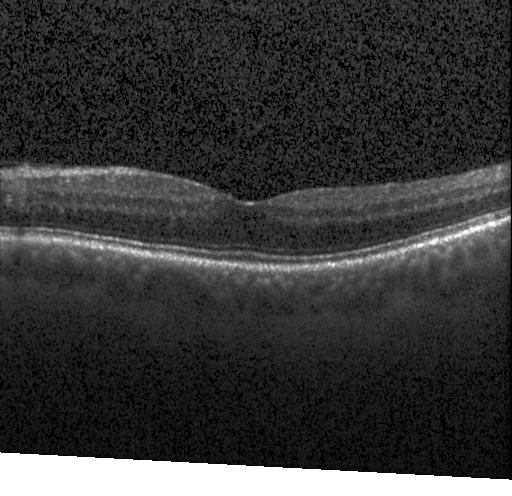

Optical coherence tomography scan.
Diagnosis: no choroidal neovascularization, diabetic macular edema, or drusen.